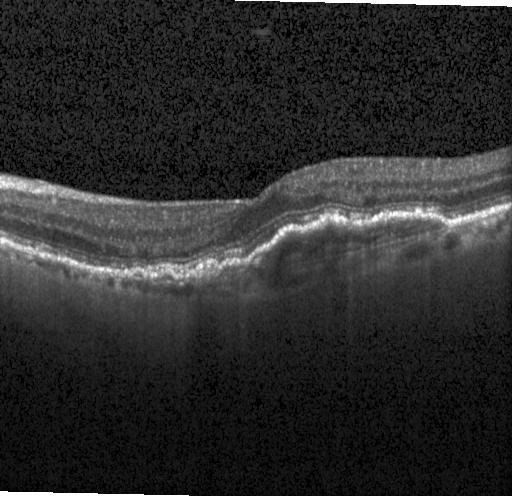 Retinal OCT B-scan
OCT finding: a choroidal neovascular membrane.